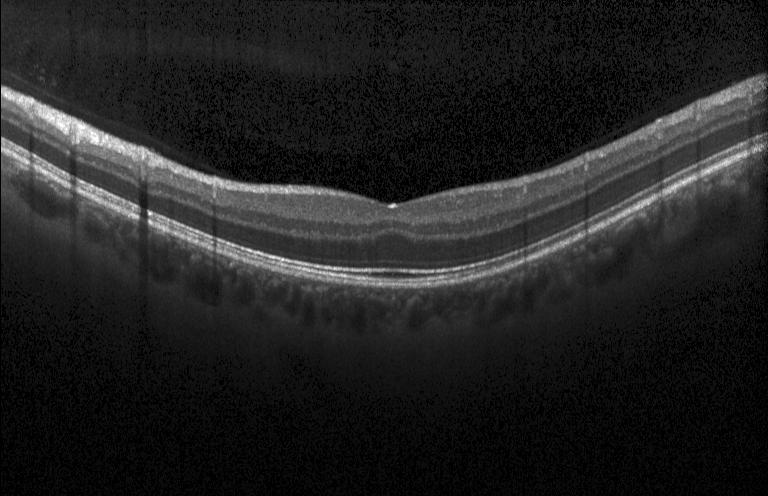 Macular scan. Instrument: Heidelberg Spectralis. OCT line scan
Finding: neither choroidal neovascularization, diabetic macular edema, nor drusen.